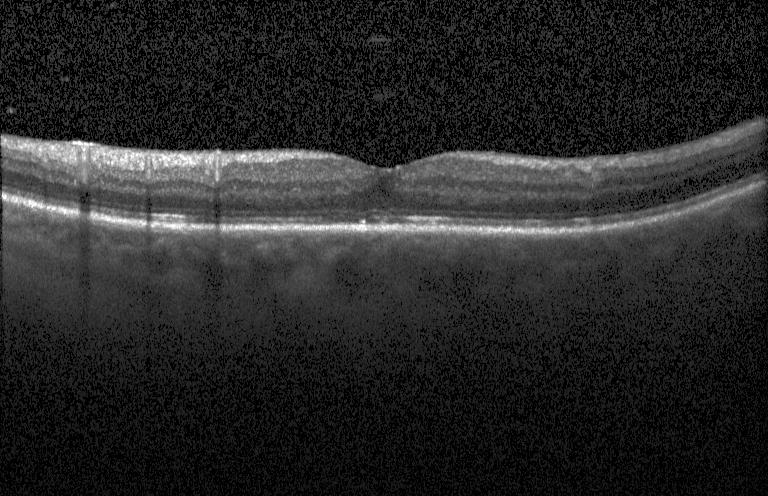 Optical coherence tomography scan.
OCT finding: no evidence of CNV, DME, or drusen.